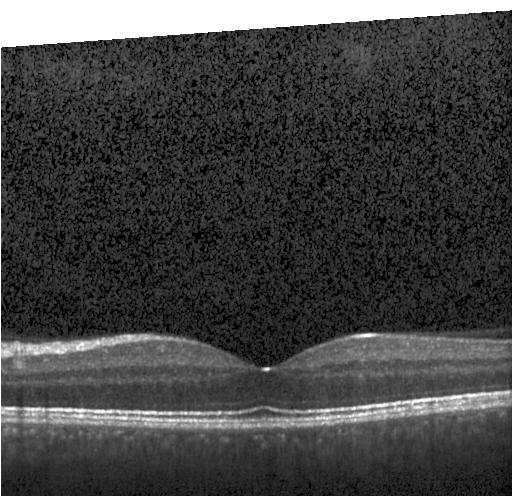
OCT B-scan — The scan shows no CNV, no DME, and no drusen.